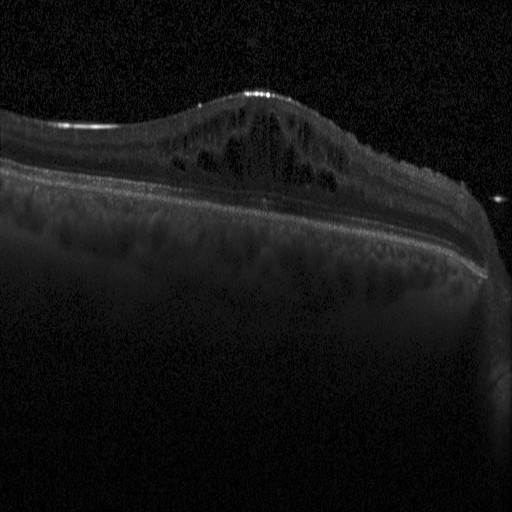
Macular OCT demonstrating DME.